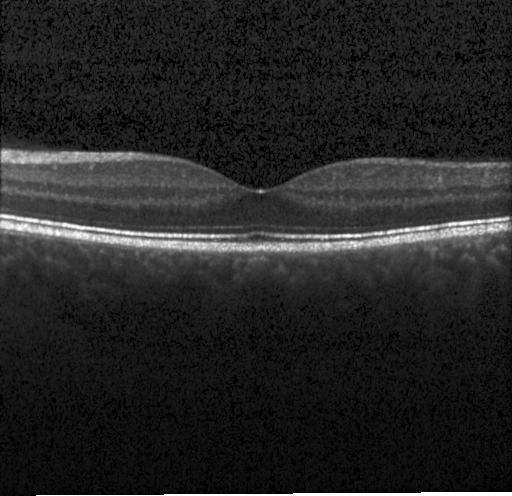
Retinal OCT cross-section — Impression: no CNV, DME, or drusen.